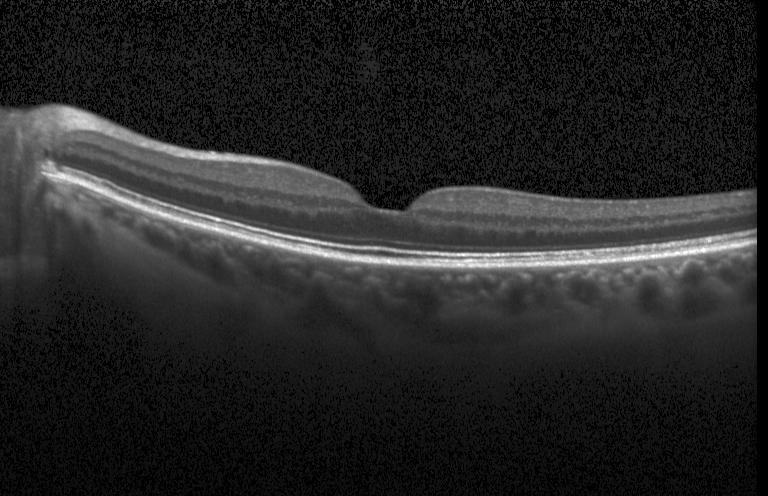 OCT B-scan · through the macula · Heidelberg Spectralis OCT system · spectral-domain OCT
No choroidal neovascularization, no diabetic macular edema, and no drusen.